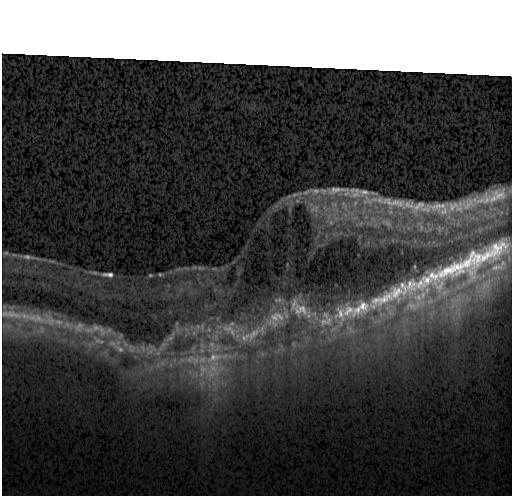
Impression: a choroidal neovascular membrane.